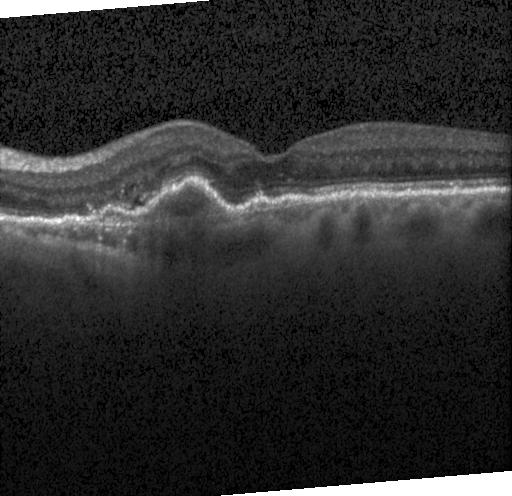 SD-OCT. Macular scan. Optical coherence tomography scan. Instrument: Heidelberg Spectralis.
Impression: CNV.